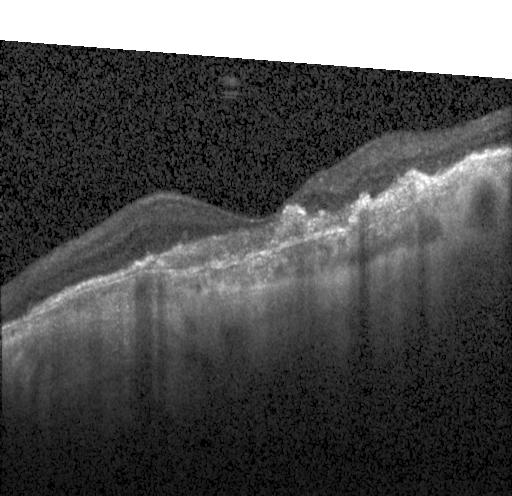

Instrument: Heidelberg Spectralis · spectral-domain OCT · through the macula · retinal OCT cross-section.
The scan shows CNV.